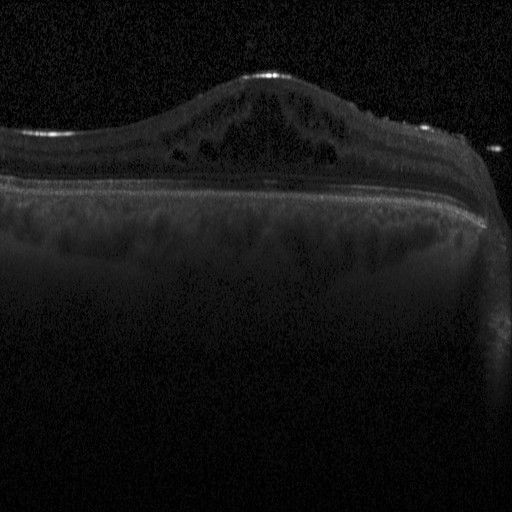

Retinal OCT cross-section showing diabetic macular edema.